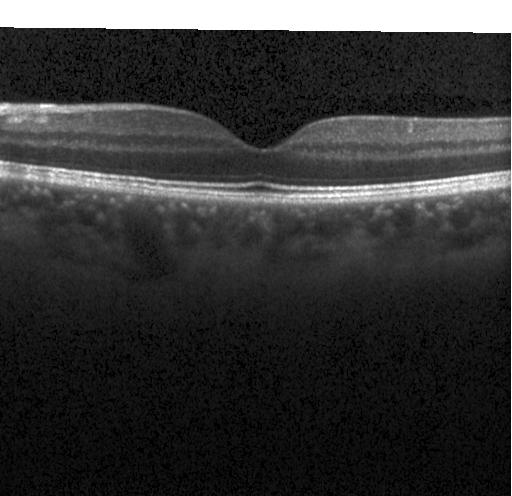 Through the macula · optical coherence tomography B-scan. This B-scan demonstrates no choroidal neovascularization, diabetic macular edema, or drusen.